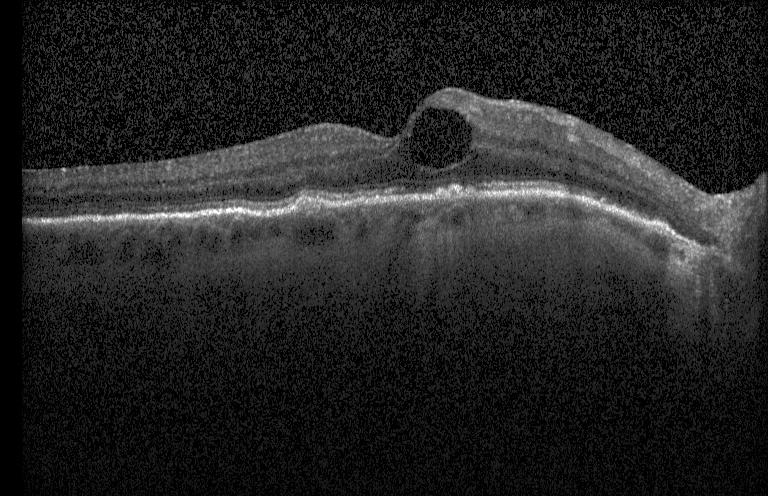 OCT B-scan. SD-OCT. Diagnosis: CNV.